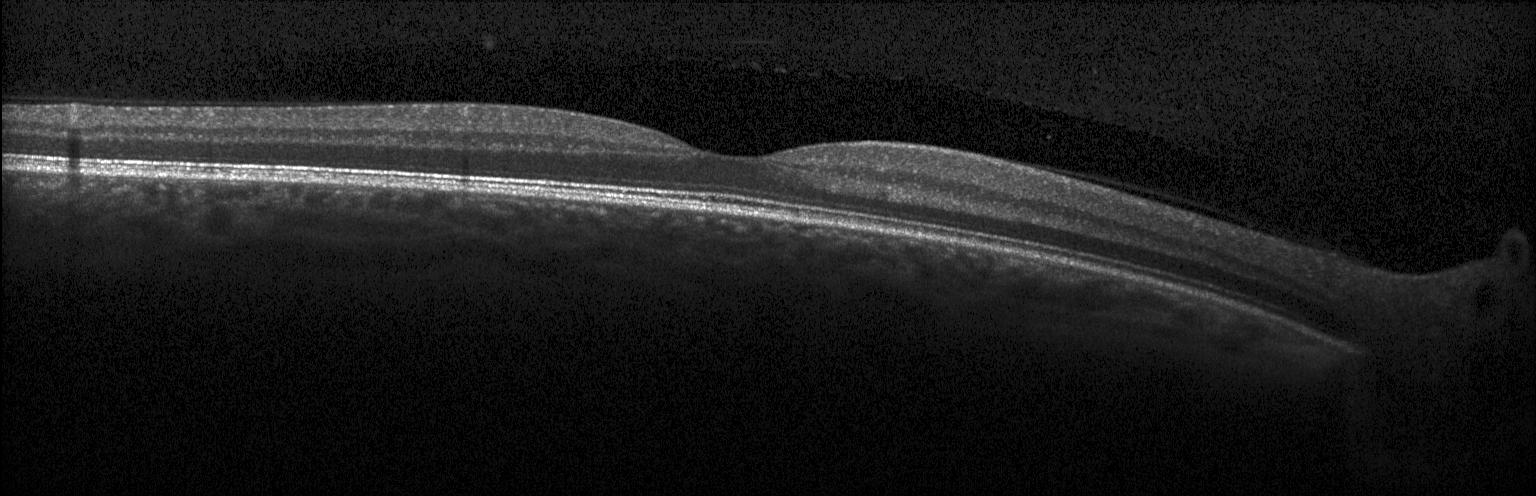
Macular OCT demonstrating no choroidal neovascularization, diabetic macular edema, or drusen.